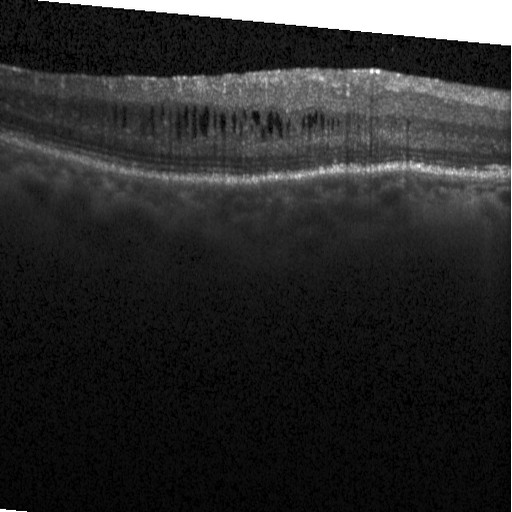

Optical coherence tomography scan. Impression: DME.